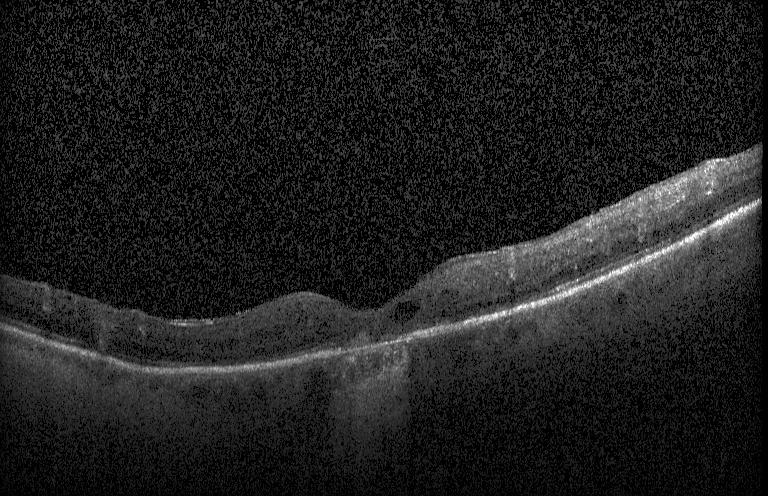

Impression: choroidal neovascularization.